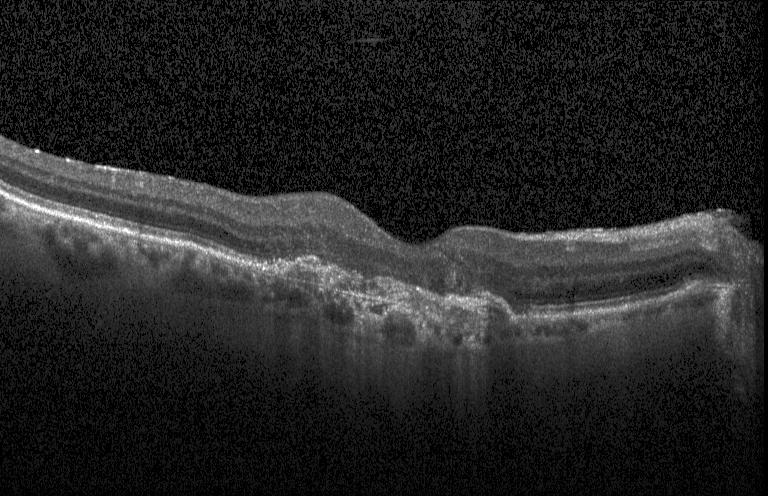 SD-OCT. Horizontal scan through the fovea. Optical coherence tomography B-scan. Diagnosis: a choroidal neovascular membrane.